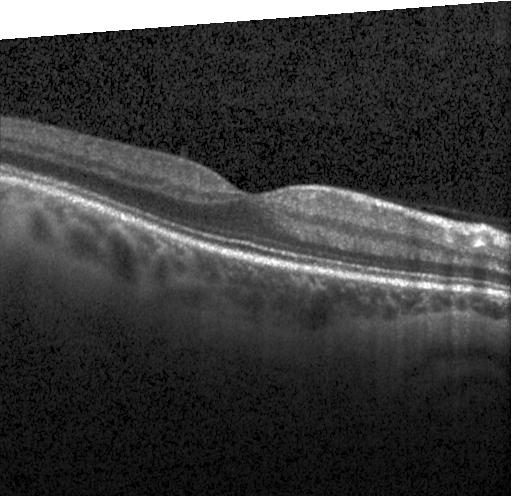
Through the macula; SD-OCT; OCT B-scan.
Dx: no evidence of choroidal neovascularization, diabetic macular edema, or drusen.